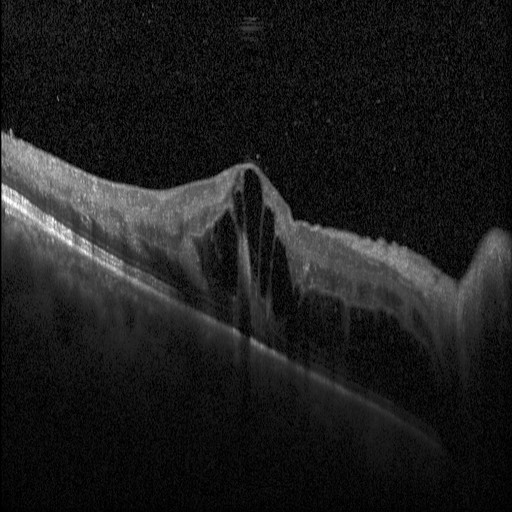 Dx: DME.